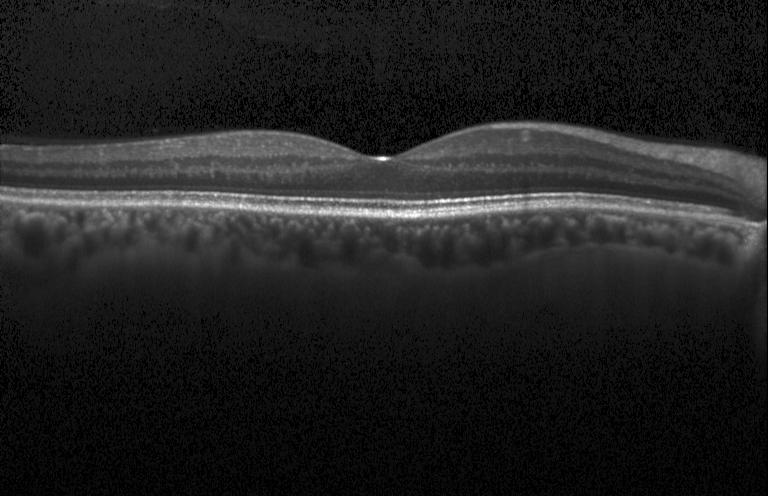

Horizontal scan through the fovea · optical coherence tomography scan · Heidelberg Spectralis
Diagnosis: no choroidal neovascularization, diabetic macular edema, or drusen.